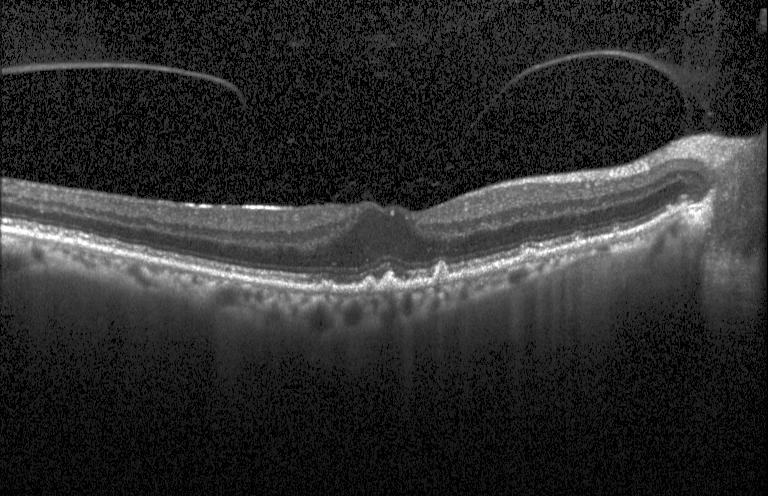

Assessment: multiple drusen.